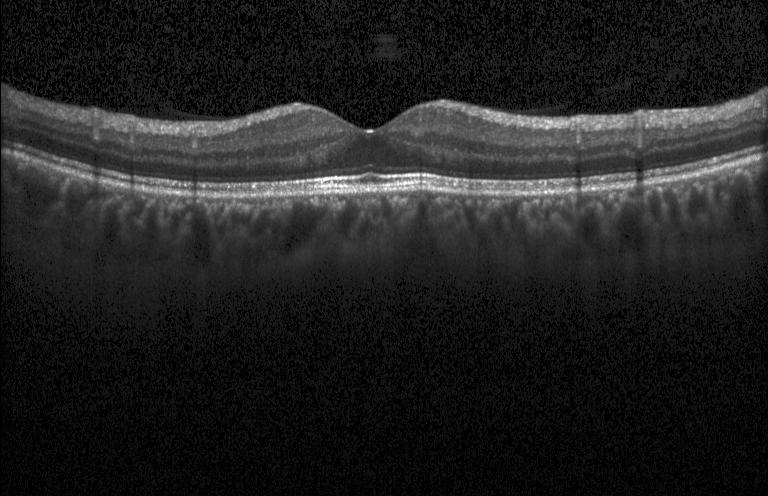
OCT scan showing no evidence of CNV, DME, or drusen.